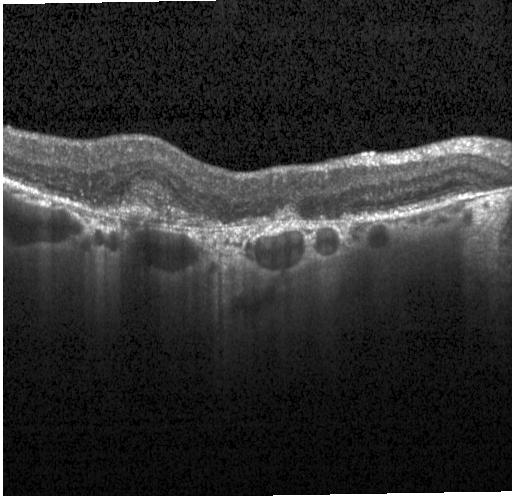 Retinal OCT cross-section. Fovea-centered.
Diagnosis: a choroidal neovascular membrane.